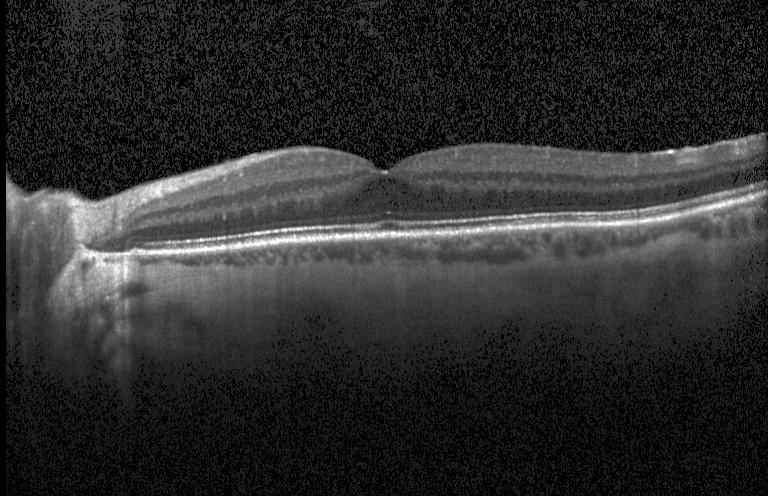

Retinal OCT B-scan · Heidelberg Spectralis · spectral-domain OCT — Diagnosis: no choroidal neovascularization, no diabetic macular edema, and no drusen.